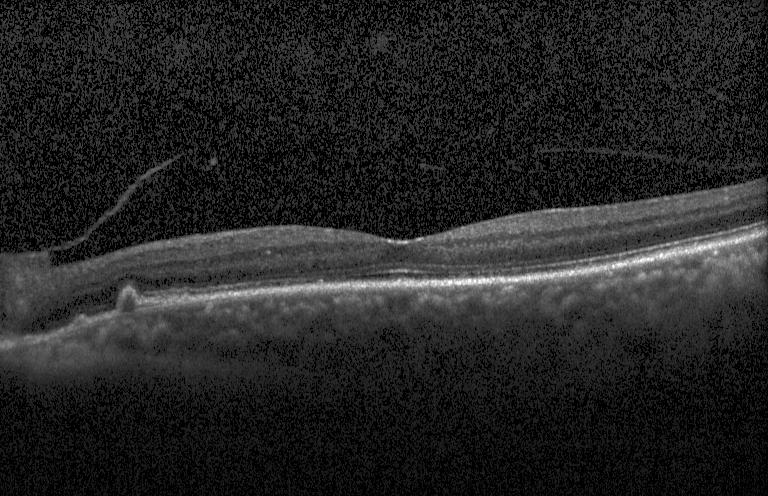

Finding: drusen.